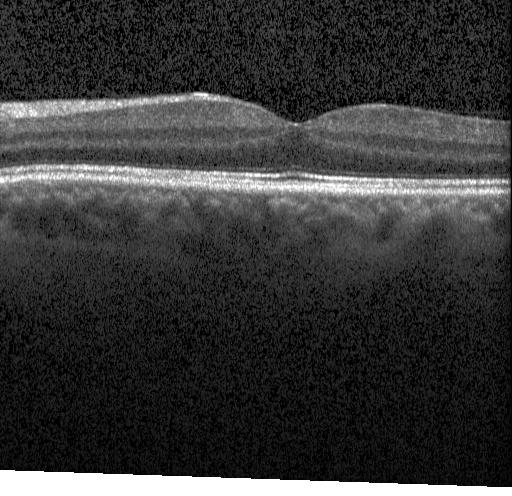
Retinal OCT cross-section
Finding: no choroidal neovascularization, no diabetic macular edema, and no drusen.